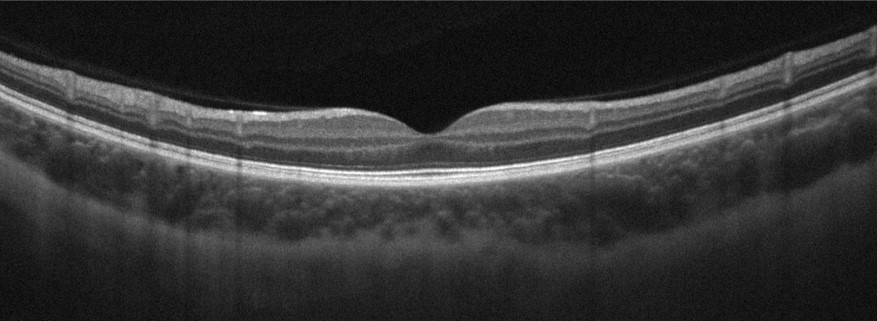
Optovue Avanti RTVue XR; retinal OCT cross-section; through the macula — Diagnosis: no evidence of AMD, DME, ERM, RAO, RVO, or VID.